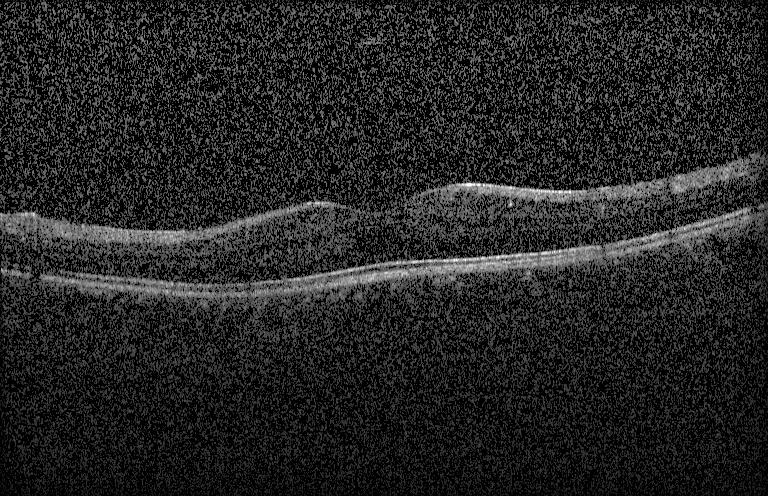 Spectral-domain OCT. Instrument: Heidelberg Spectralis. Retinal OCT cross-section — Impression: no choroidal neovascularization, diabetic macular edema, or drusen.